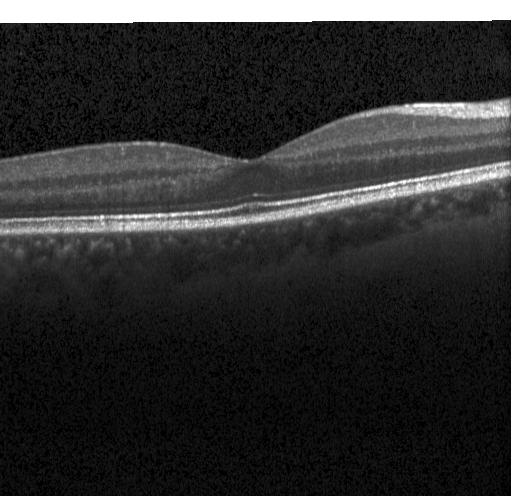
Macular OCT: no evidence of choroidal neovascularization, diabetic macular edema, or drusen.